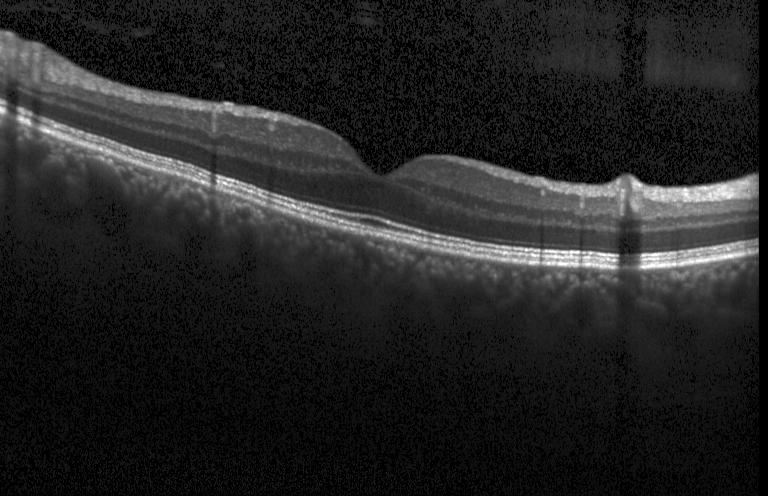
OCT line scan — Finding: neither choroidal neovascularization, diabetic macular edema, nor drusen.